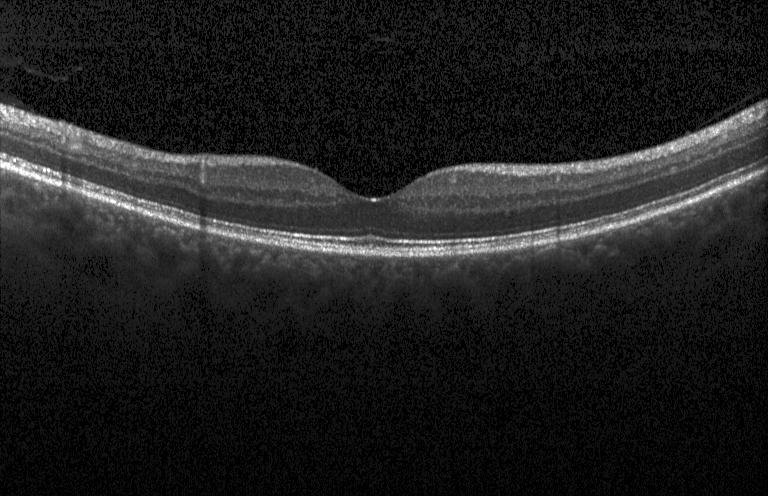
SD-OCT, OCT B-scan, through the macula — No choroidal neovascularization, diabetic macular edema, or drusen.